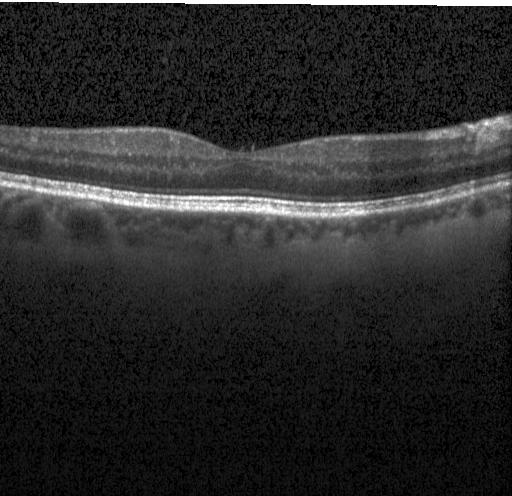
Optical coherence tomography scan.
The scan shows no evidence of CNV, DME, or drusen.